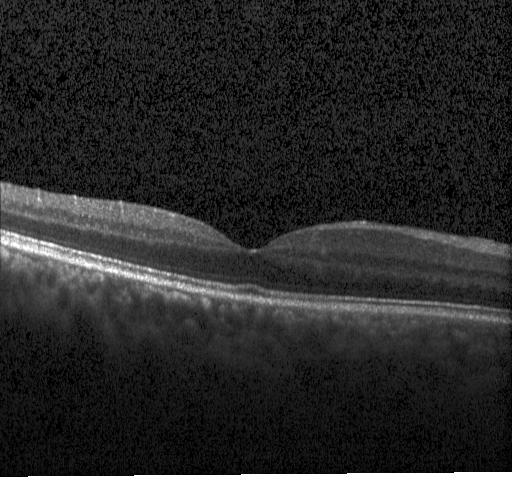
OCT B-scan · through the macula. OCT finding: no choroidal neovascularization, no diabetic macular edema, and no drusen.